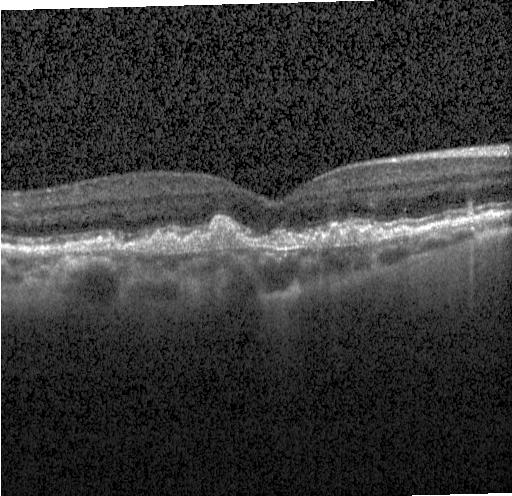
Acquired on a Heidelberg Spectralis, spectral-domain optical coherence tomography, retinal OCT B-scan.
This B-scan demonstrates a choroidal neovascular membrane.